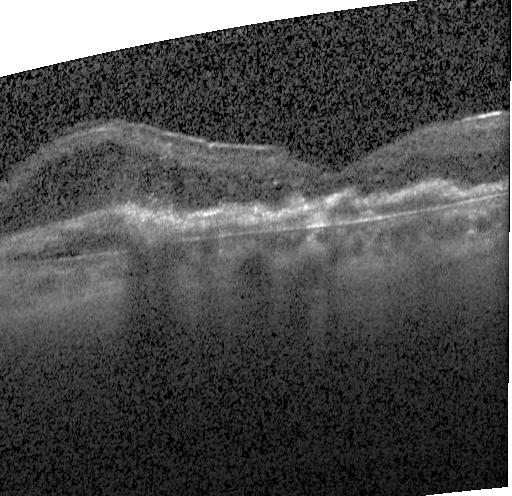
Optical coherence tomography B-scan; spectral-domain optical coherence tomography; horizontal scan through the fovea; Heidelberg Spectralis. Diagnosis: CNV.